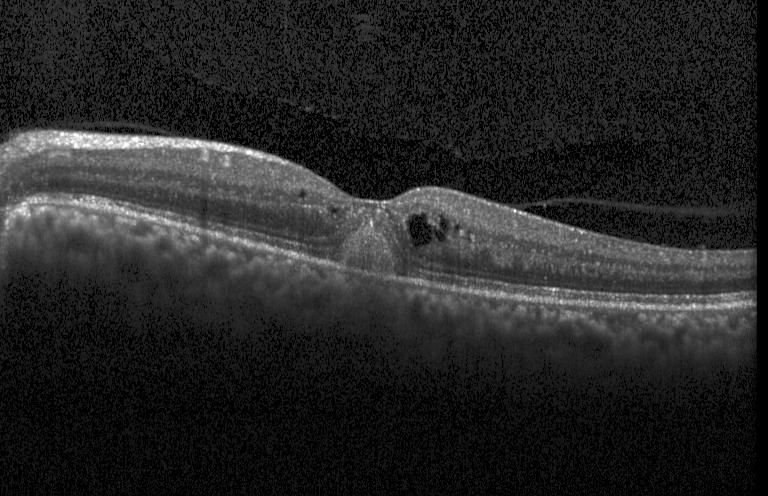 Spectral-domain optical coherence tomography; acquired on a Heidelberg Spectralis; fovea-centered; optical coherence tomography scan — Impression: a choroidal neovascular membrane.